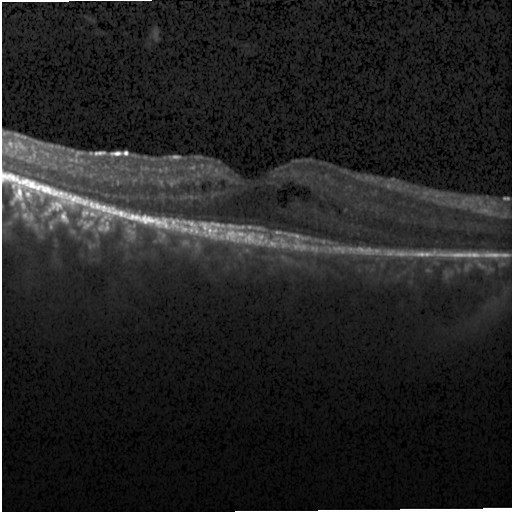
Through the macula; OCT line scan; spectral-domain OCT.
Dx: diabetic macular edema (DME).